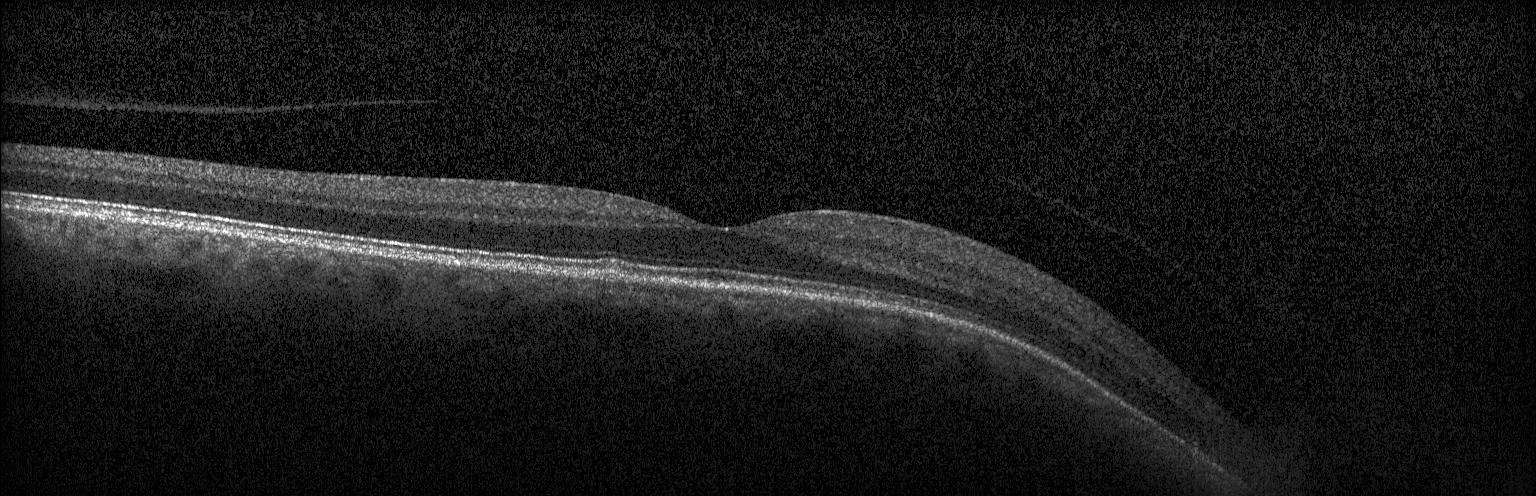

Macular OCT demonstrating no evidence of choroidal neovascularization, diabetic macular edema, or drusen.